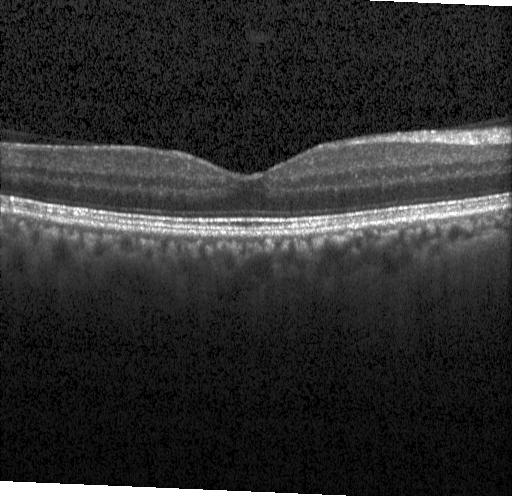 Optical coherence tomography scan. Heidelberg Spectralis OCT system. Spectral-domain OCT. Fovea-centered — Finding: no evidence of CNV, DME, or drusen.